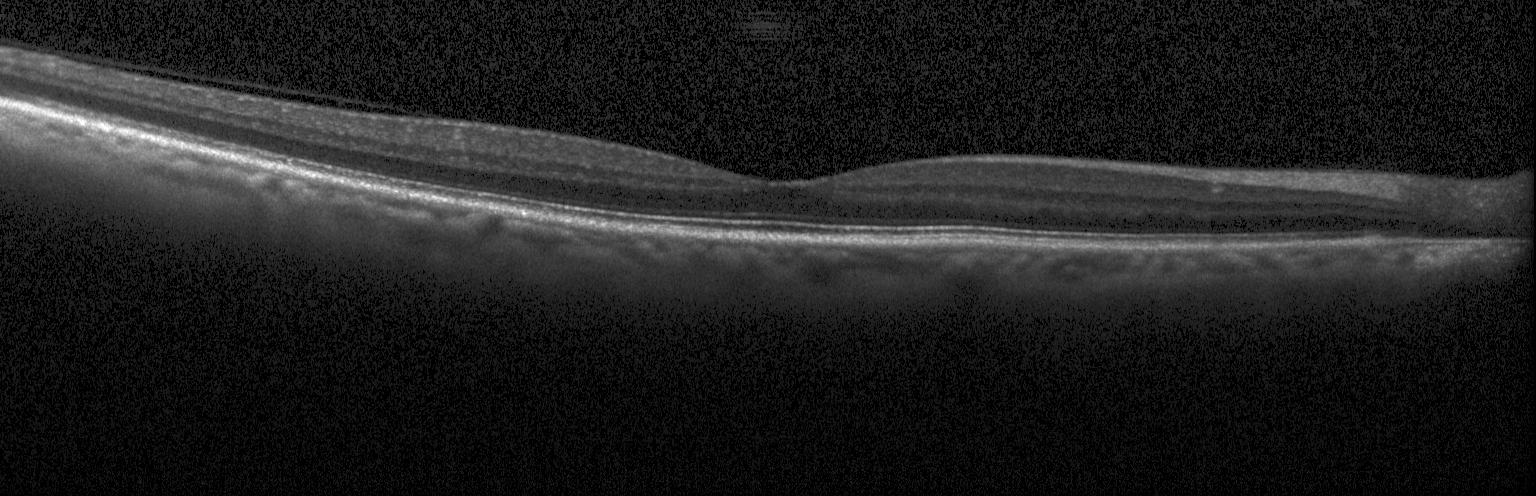
Dx: neither choroidal neovascularization, diabetic macular edema, nor drusen.